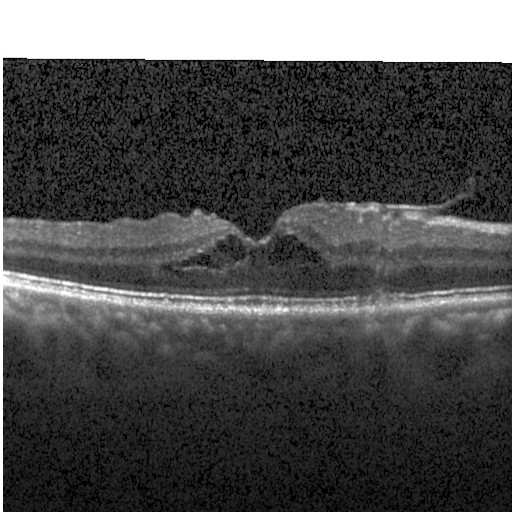 Retinal OCT B-scan, spectral-domain optical coherence tomography, horizontal scan through the fovea.
This B-scan demonstrates diabetic macular edema.